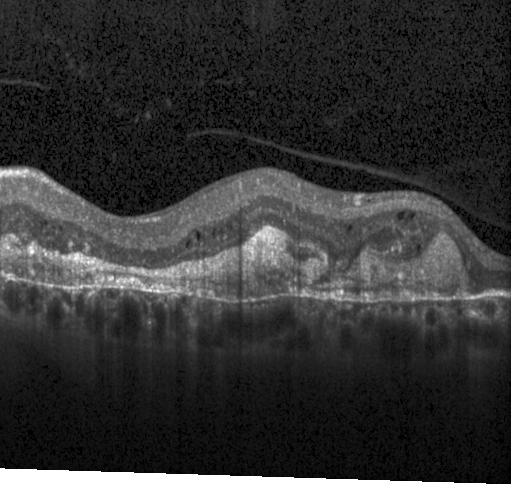

Instrument: Heidelberg Spectralis; SD-OCT; centered on the fovea; optical coherence tomography B-scan. This B-scan demonstrates CNV.